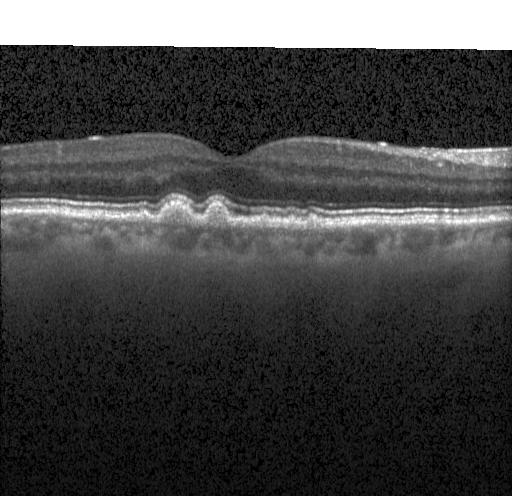 OCT line scan · spectral-domain OCT
OCT finding: sub-RPE drusenoid deposits.